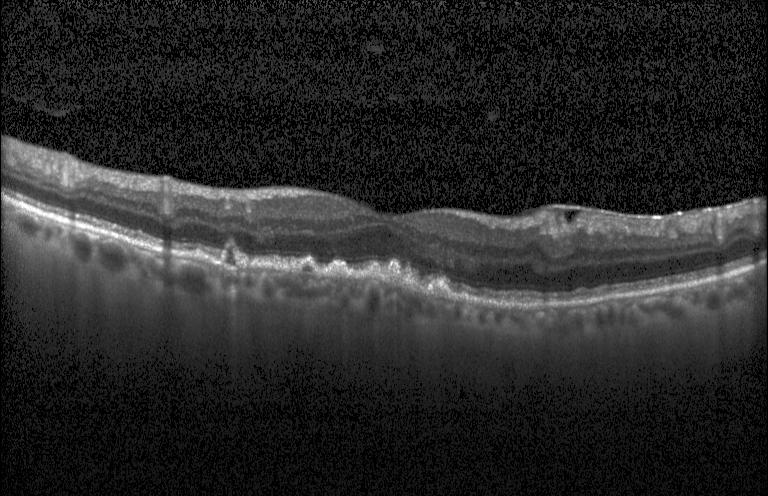
Acquired on a Heidelberg Spectralis, retinal OCT cross-section, spectral-domain optical coherence tomography.
Impression: a choroidal neovascular membrane.